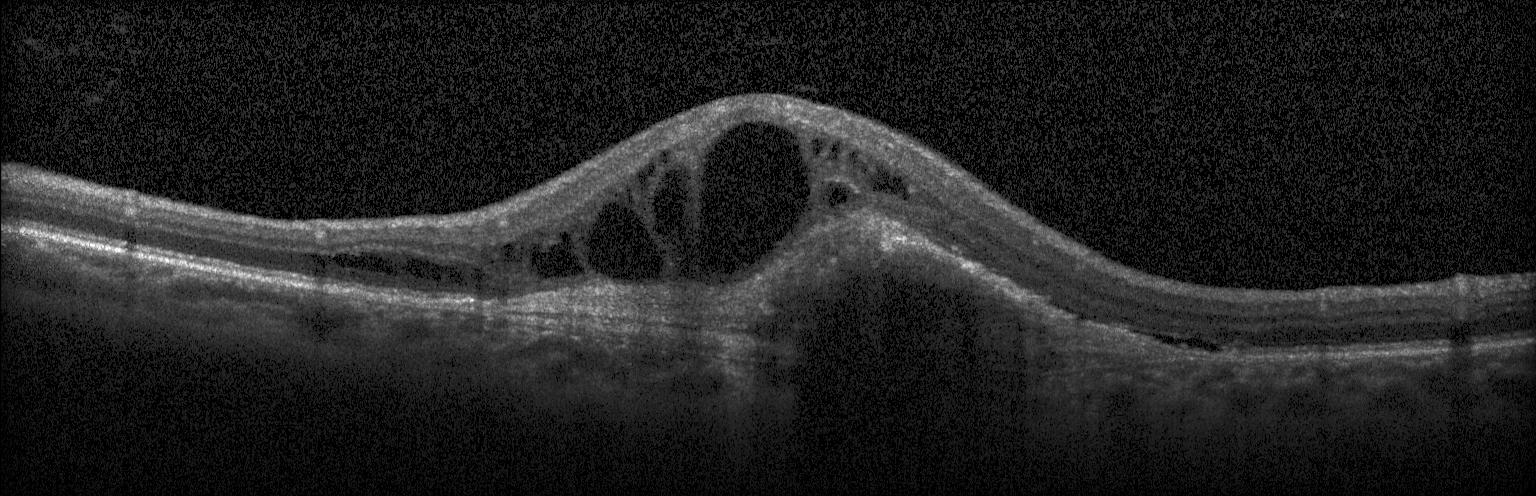 OCT line scan — Diagnosis: choroidal neovascularization.